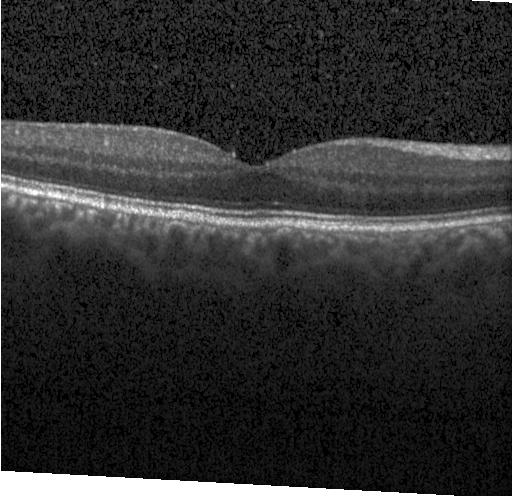
Impression: neither CNV, DME, nor drusen.